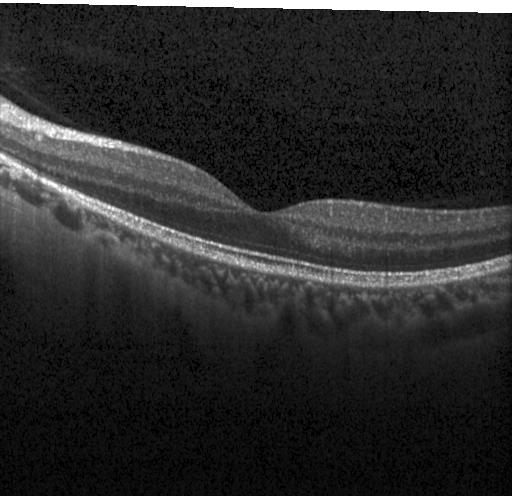
OCT line scan. Spectral-domain optical coherence tomography — Dx: no evidence of choroidal neovascularization, diabetic macular edema, or drusen.